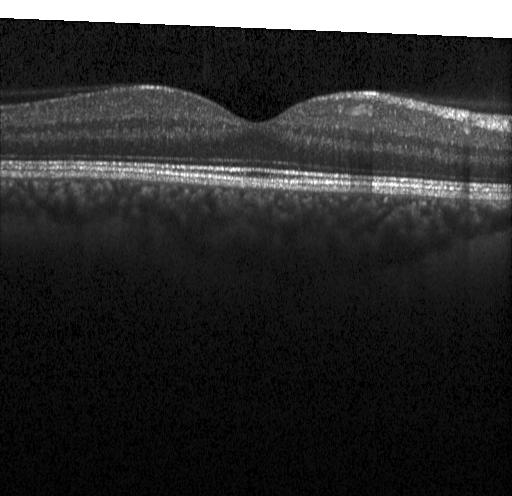 Optical coherence tomography B-scan. Impression: no choroidal neovascularization, no diabetic macular edema, and no drusen.